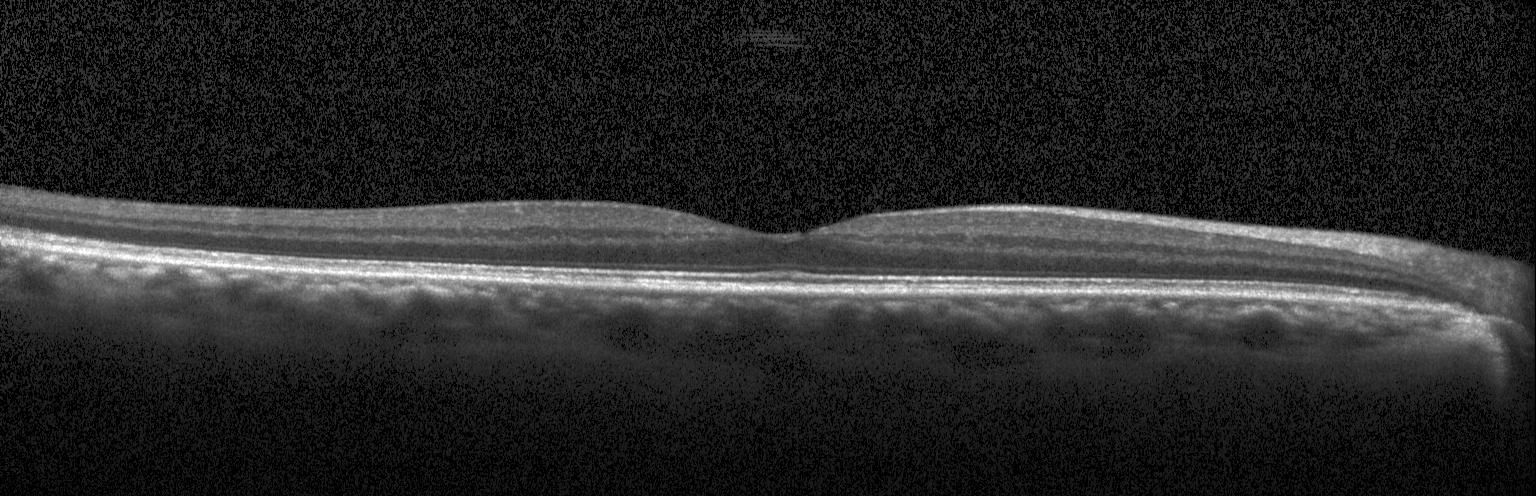

Optical coherence tomography B-scan — This B-scan demonstrates neither choroidal neovascularization, diabetic macular edema, nor drusen.